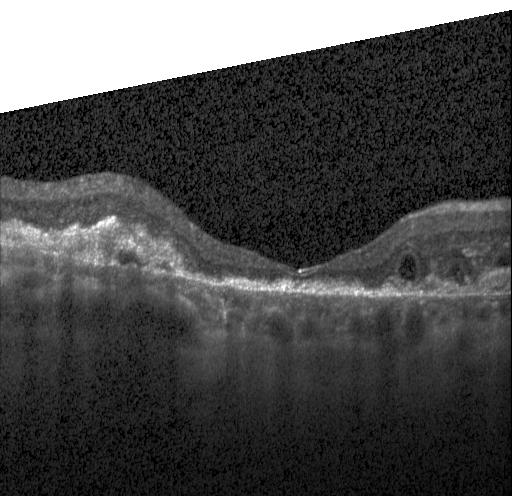 Optical coherence tomography scan — Diagnosis: a choroidal neovascular membrane.